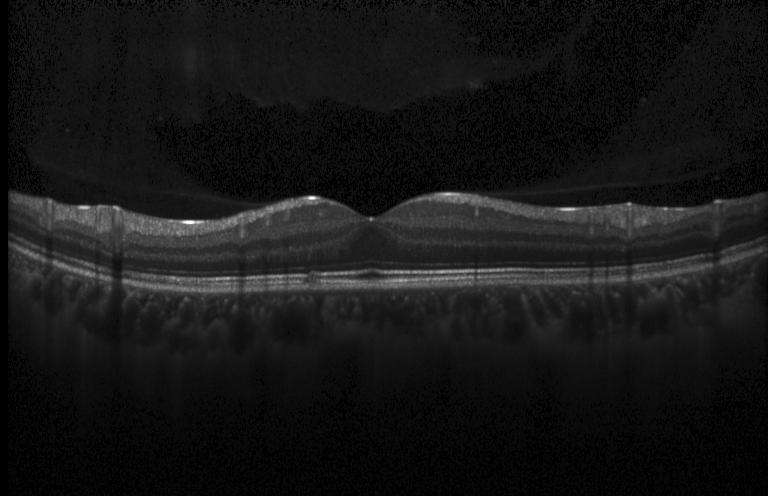
Instrument: Heidelberg Spectralis. Through the macula. Spectral-domain OCT. Optical coherence tomography scan — Finding: no CNV, no DME, and no drusen.